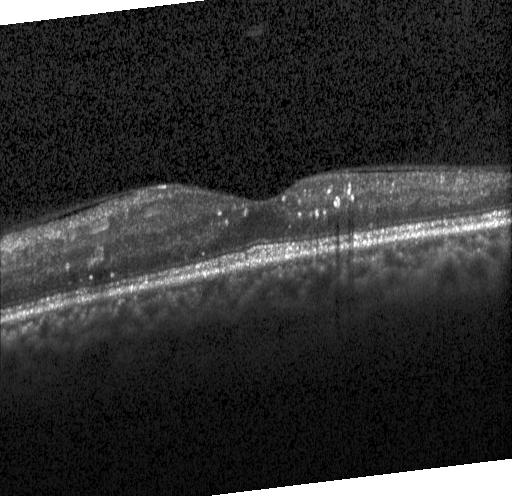 Optical coherence tomography B-scan. Fovea-centered. Spectral-domain OCT. Impression: diabetic macular edema.